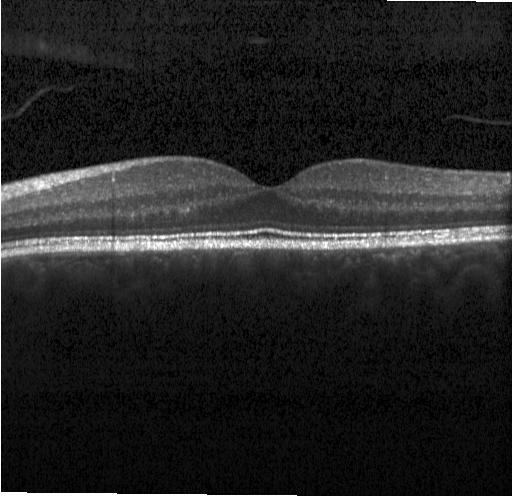
Macular scan, optical coherence tomography scan, Heidelberg Spectralis OCT system.
The scan shows no choroidal neovascularization, no diabetic macular edema, and no drusen.